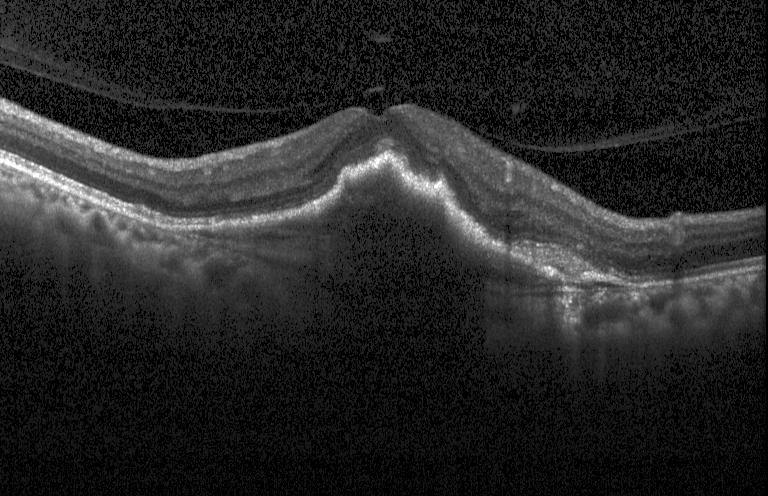

Retinal OCT cross-section showing CNV.